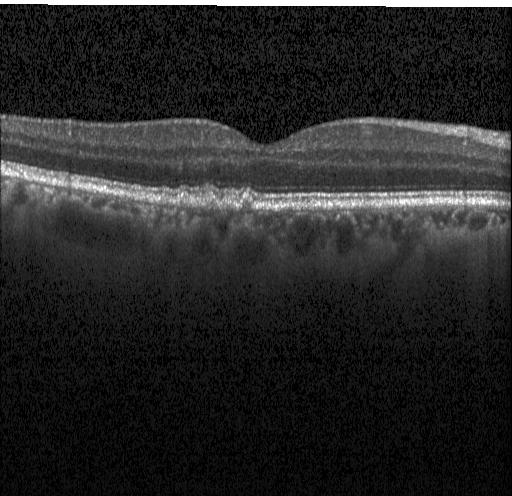

Finding: drusen.